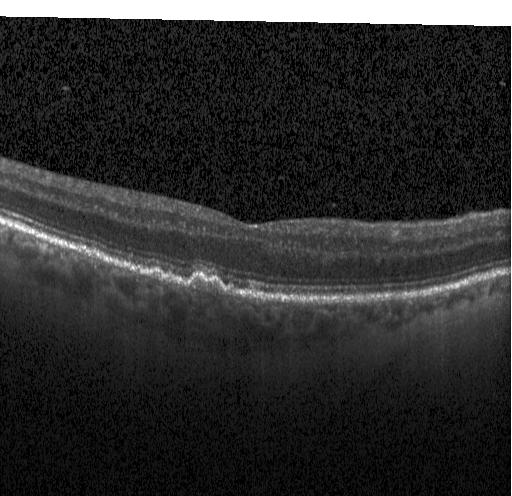

Heidelberg Spectralis · OCT B-scan · fovea-centered
This B-scan demonstrates sub-RPE drusenoid deposits.